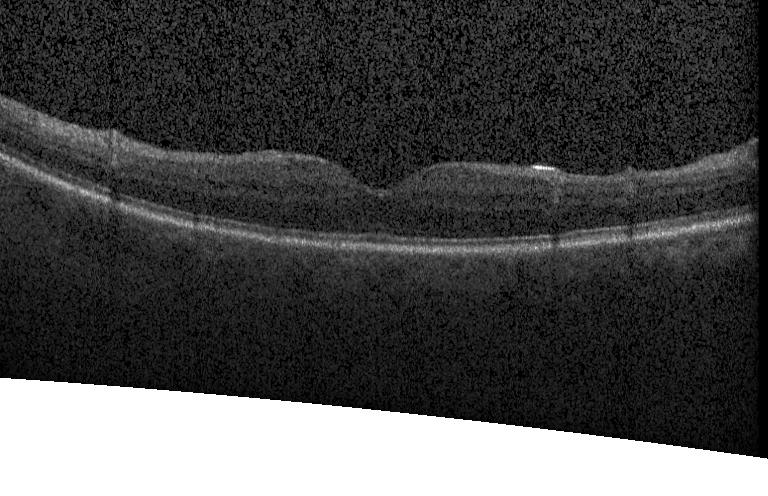 Optical coherence tomography scan; SD-OCT. Impression: no evidence of choroidal neovascularization, diabetic macular edema, or drusen.